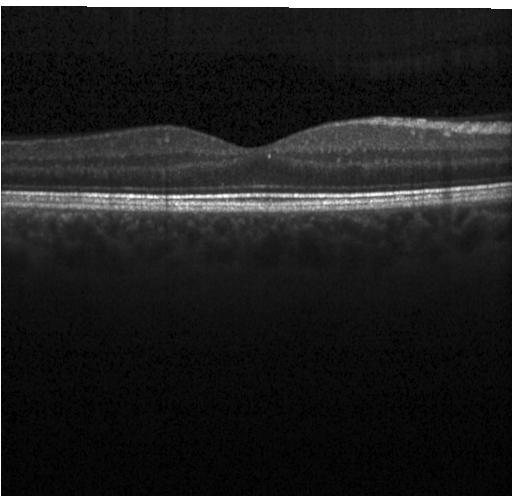

Heidelberg Spectralis, horizontal scan through the fovea, SD-OCT, optical coherence tomography scan. No choroidal neovascularization, no diabetic macular edema, and no drusen.